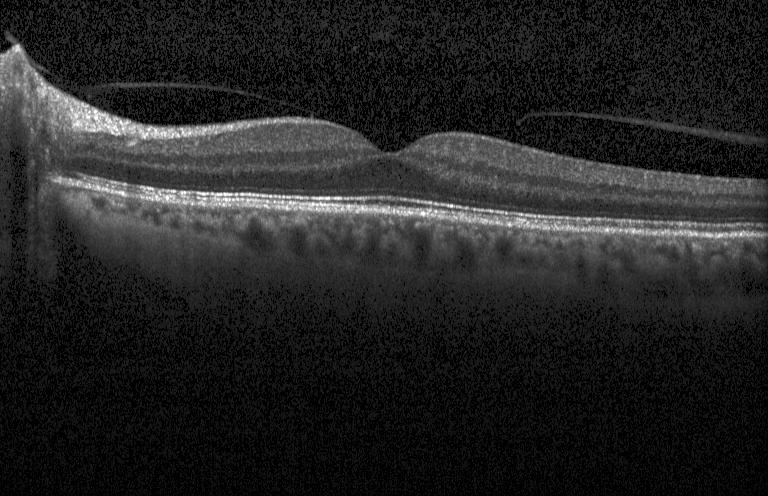
Through the macula; optical coherence tomography B-scan; SD-OCT; Heidelberg Spectralis — Diagnosis: no choroidal neovascularization, no diabetic macular edema, and no drusen.